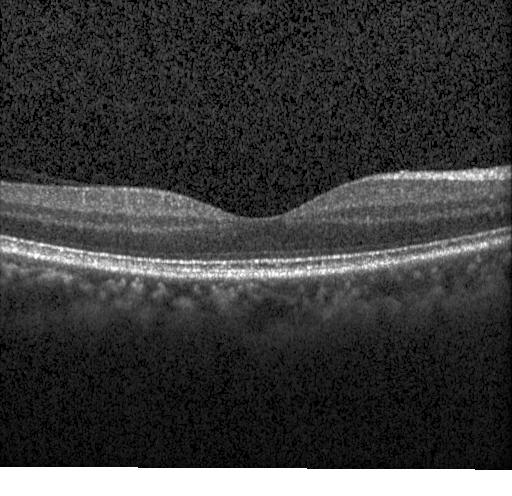 No choroidal neovascularization, no diabetic macular edema, and no drusen.